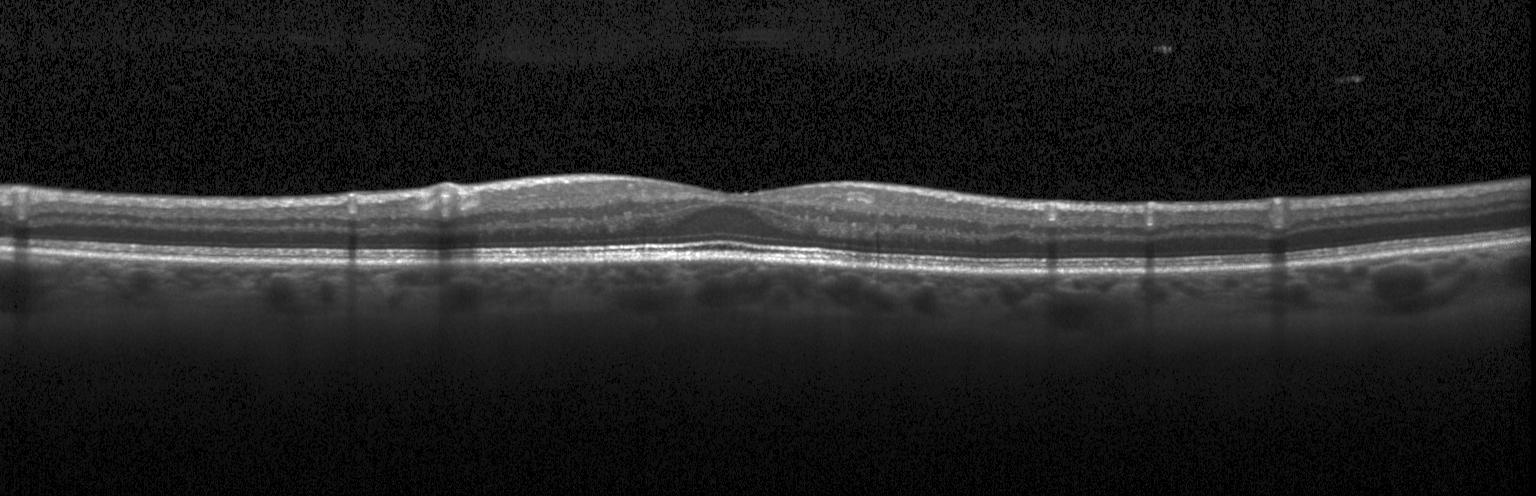
Dx: no choroidal neovascularization, no diabetic macular edema, and no drusen.